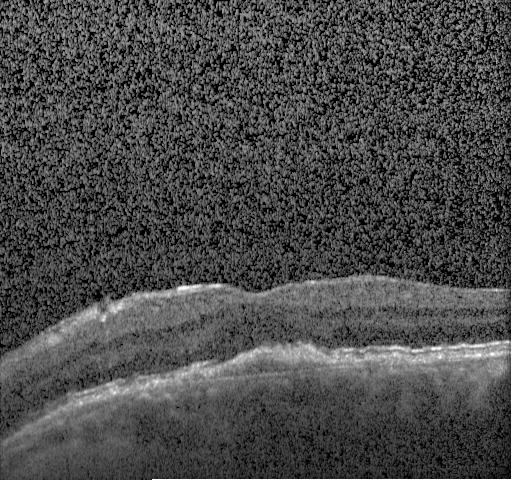 Acquired on a Heidelberg Spectralis; optical coherence tomography scan.
The scan shows CNV.